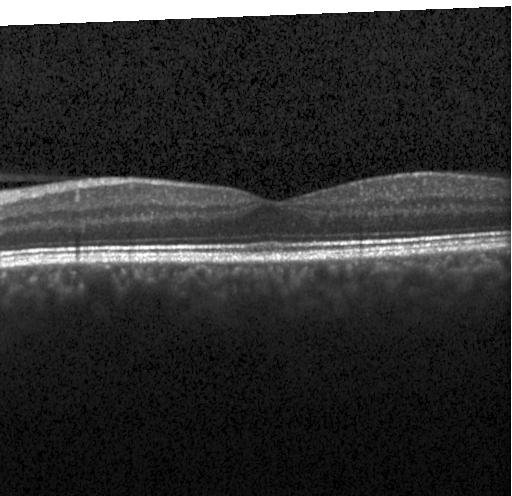

OCT B-scan — This B-scan demonstrates neither choroidal neovascularization, diabetic macular edema, nor drusen.